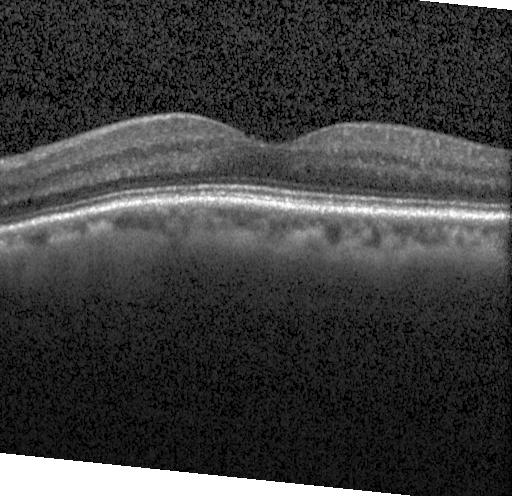
Optical coherence tomography scan. Impression: neither choroidal neovascularization, diabetic macular edema, nor drusen.